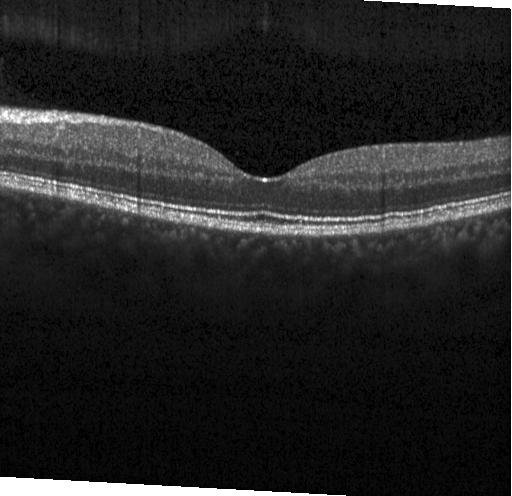
Retinal OCT cross-section showing no evidence of choroidal neovascularization, diabetic macular edema, or drusen.